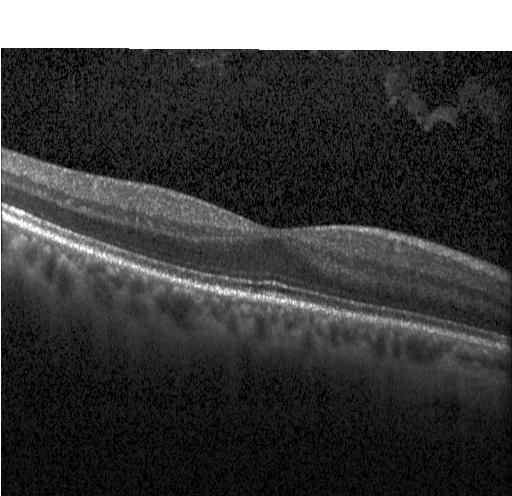
Optical coherence tomography B-scan. OCT finding: no choroidal neovascularization, diabetic macular edema, or drusen.